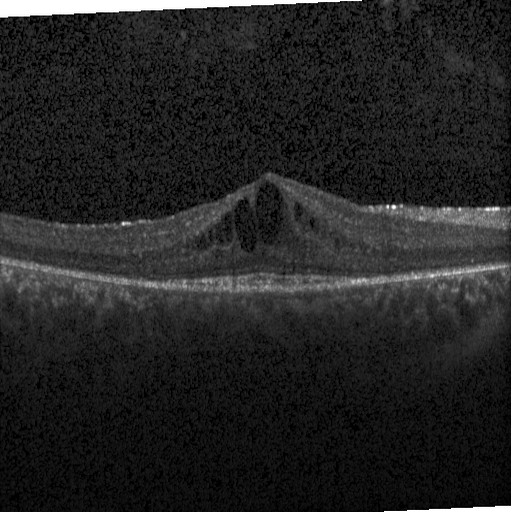
Macular OCT demonstrating DME.